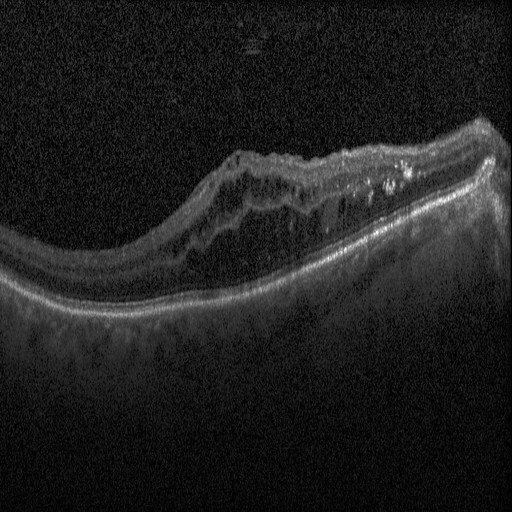

Instrument: Heidelberg Spectralis; centered on the fovea; retinal OCT cross-section — The scan shows diabetic macular edema.